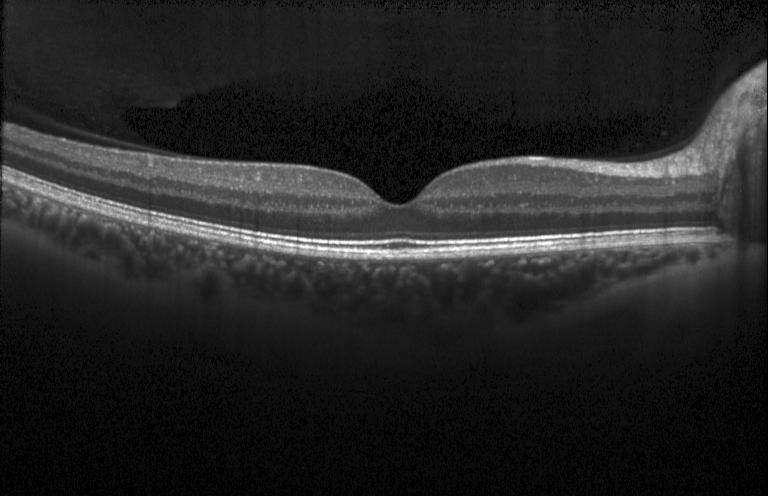
The scan shows no choroidal neovascularization, no diabetic macular edema, and no drusen.